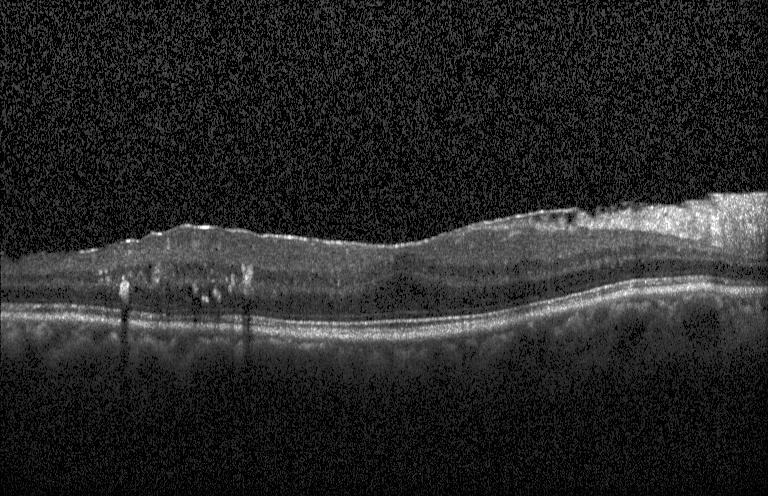 Impression: diabetic macular edema.